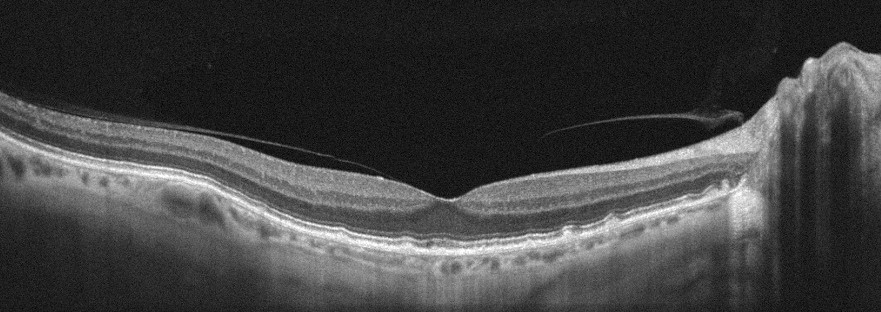

Macular OCT: AMD.